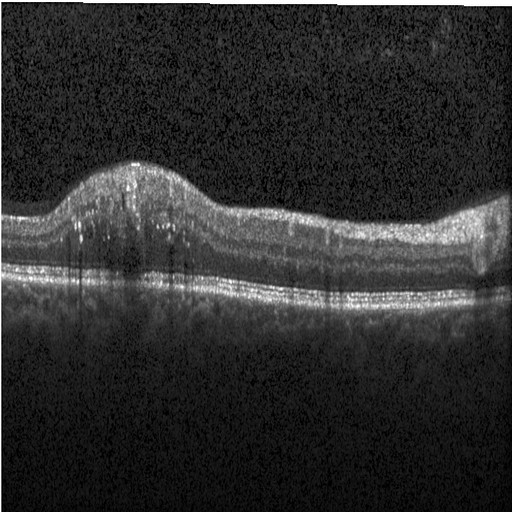 Optical coherence tomography B-scan · spectral-domain OCT.
This B-scan demonstrates diabetic macular edema.